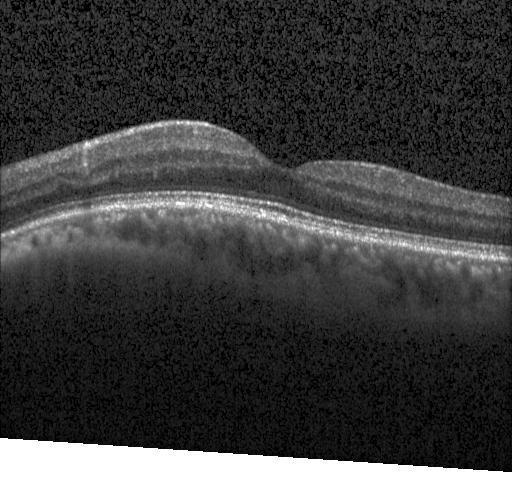
Impression: no evidence of CNV, DME, or drusen.